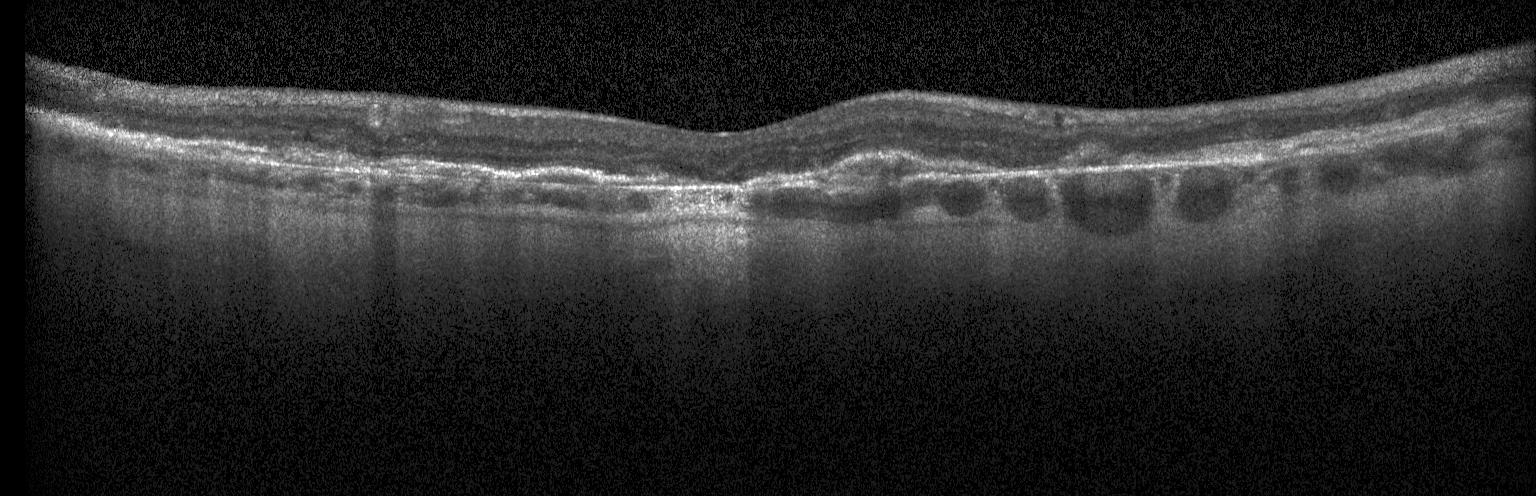

Instrument: Heidelberg Spectralis · through the macula · retinal OCT cross-section
Finding: choroidal neovascularization (CNV).